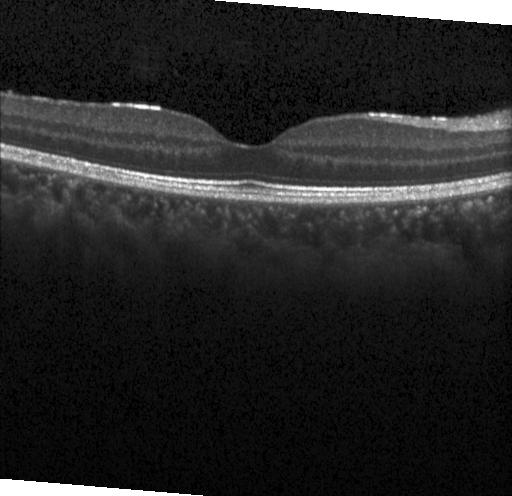 SD-OCT; retinal OCT cross-section; horizontal scan through the fovea; Heidelberg Spectralis OCT system — The scan shows neither choroidal neovascularization, diabetic macular edema, nor drusen.